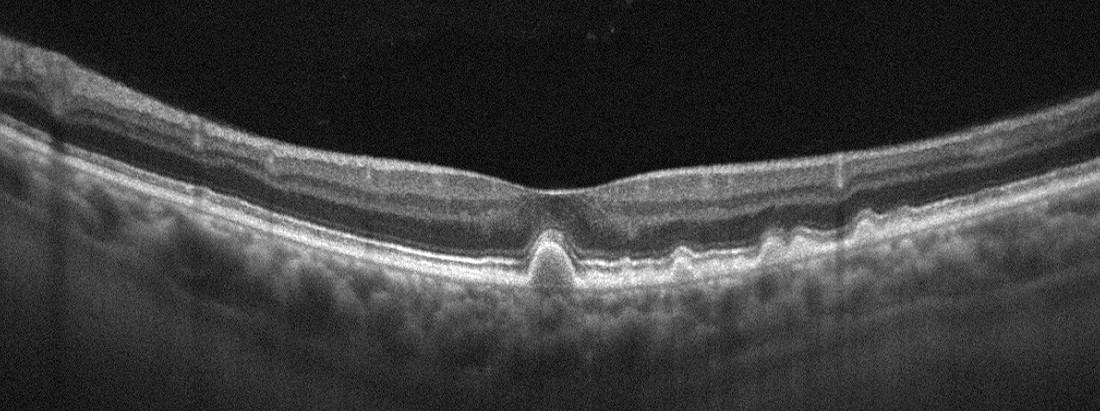

Retinal OCT cross-section.
This B-scan demonstrates AMD.